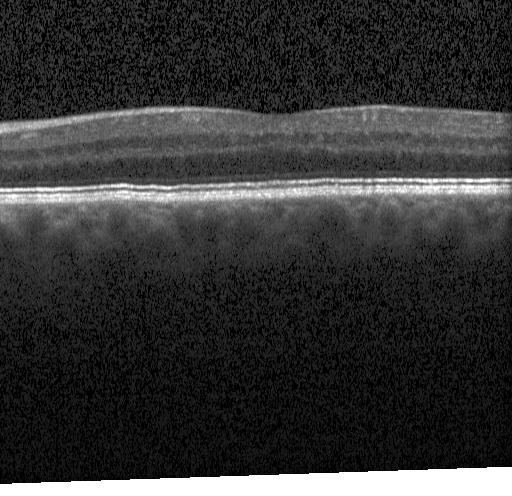
OCT B-scan — Finding: no evidence of choroidal neovascularization, diabetic macular edema, or drusen.